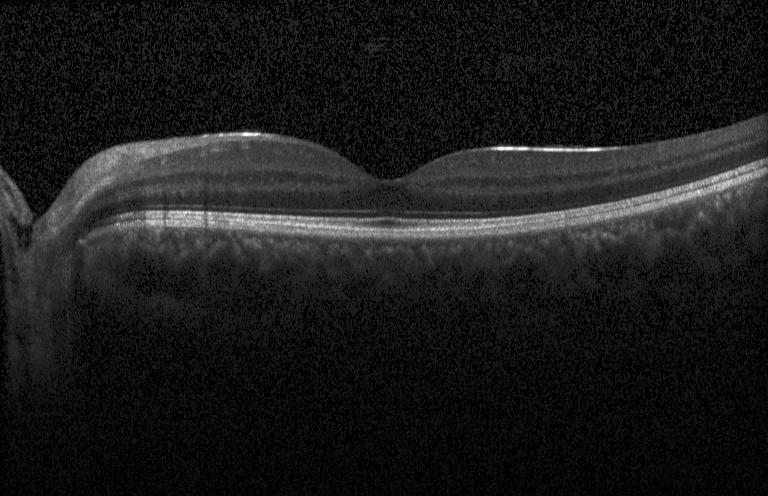 Dx: no choroidal neovascularization, diabetic macular edema, or drusen.